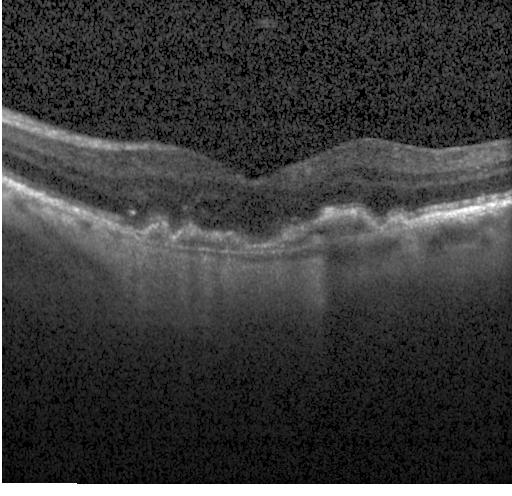

OCT B-scan. Centered on the fovea. Spectral-domain optical coherence tomography
Choroidal neovascularization.